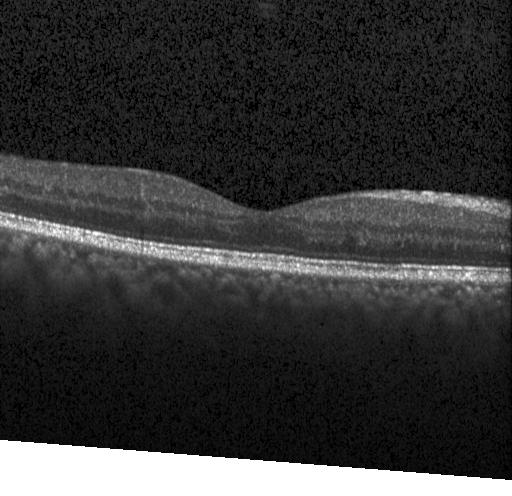

Optical coherence tomography scan, horizontal scan through the fovea, instrument: Heidelberg Spectralis, spectral-domain OCT.
Diagnosis: no evidence of choroidal neovascularization, diabetic macular edema, or drusen.